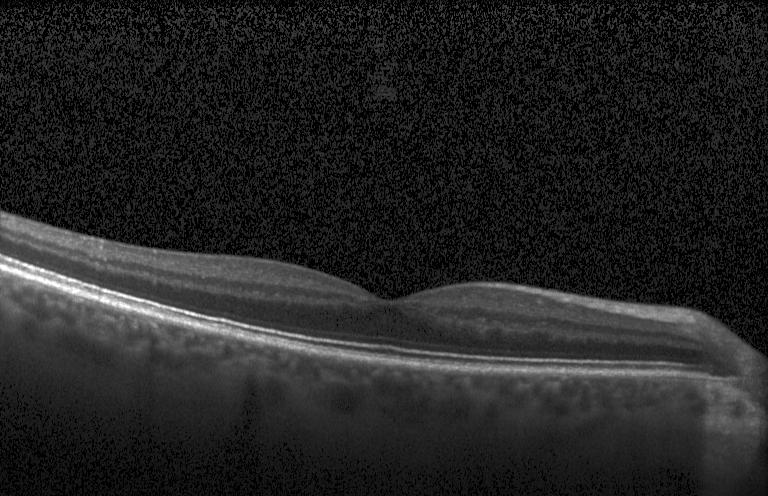

Finding: no evidence of choroidal neovascularization, diabetic macular edema, or drusen.